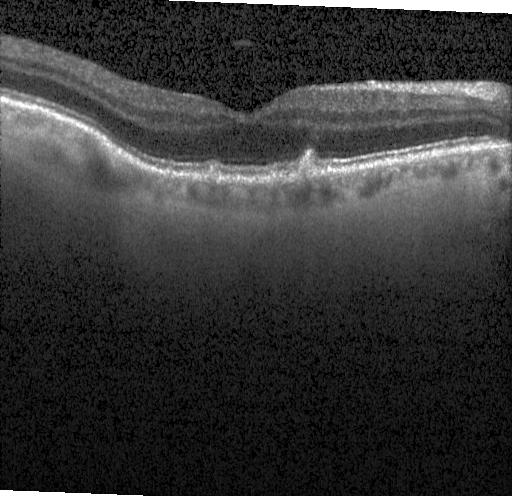 Diagnosis: sub-RPE drusenoid deposits.